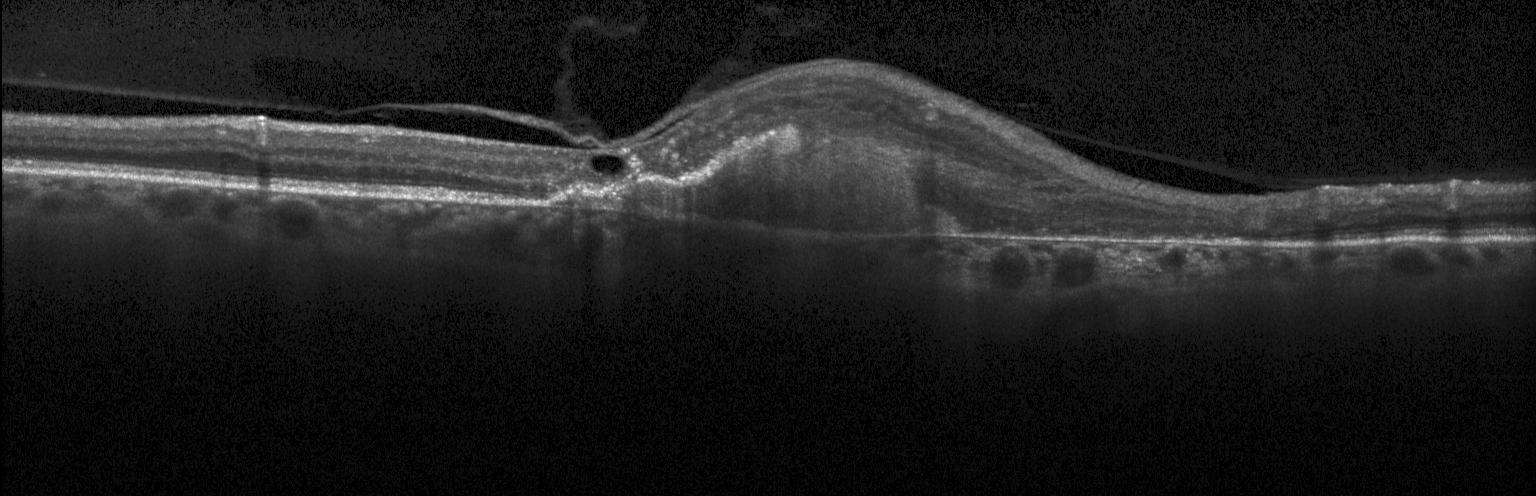 Dx: a choroidal neovascular membrane.